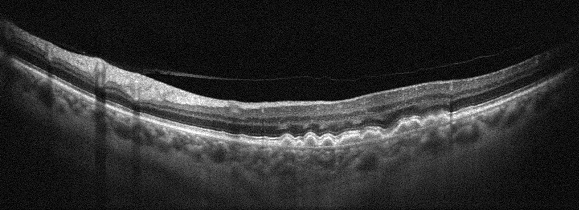

Instrument: Optovue Avanti RTVue XR; retinal OCT B-scan; through the macula.
Dx: age-related macular degeneration (AMD).